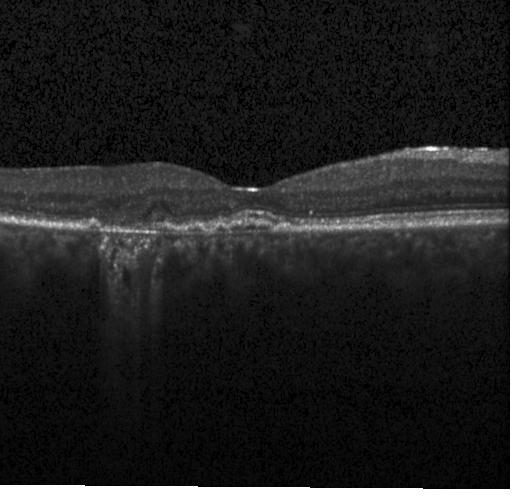 OCT B-scan, centered on the fovea, acquired on a Heidelberg Spectralis, SD-OCT
Finding: choroidal neovascularization (CNV).